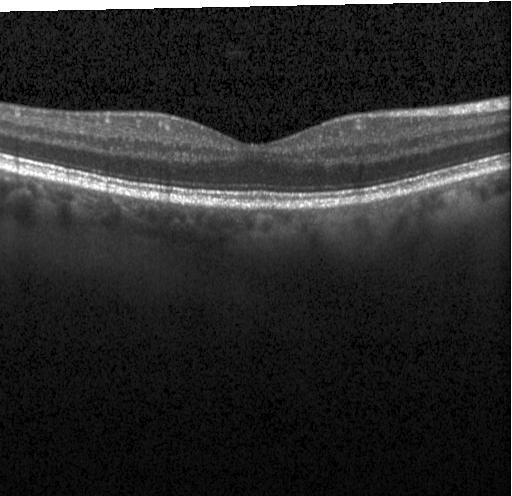
OCT line scan
Impression: no evidence of CNV, DME, or drusen.